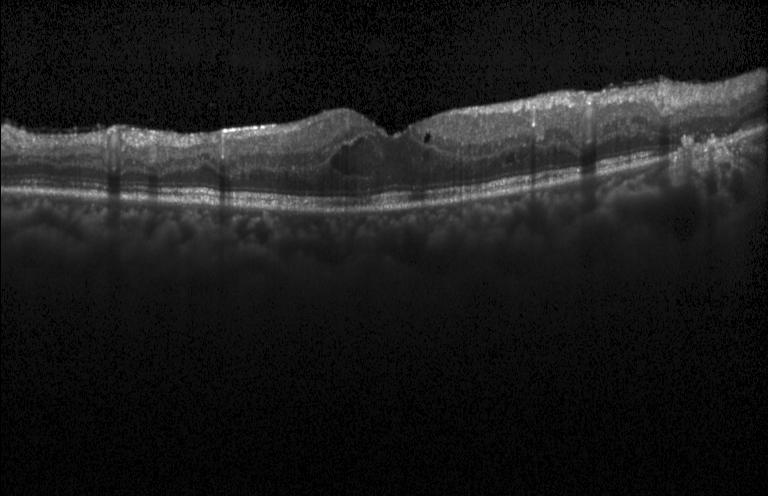
OCT B-scan; macular scan
Dx: DME.